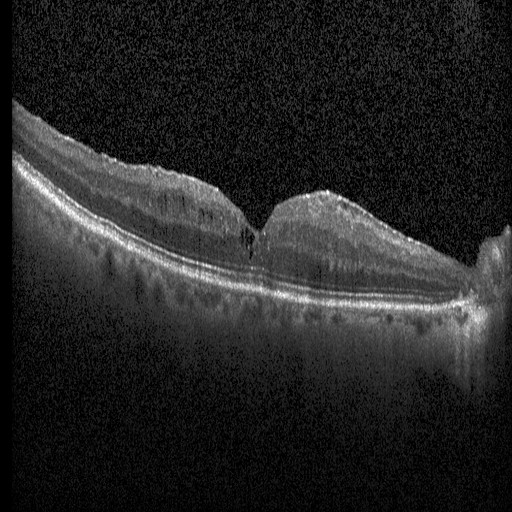

Finding: diabetic macular edema (DME).